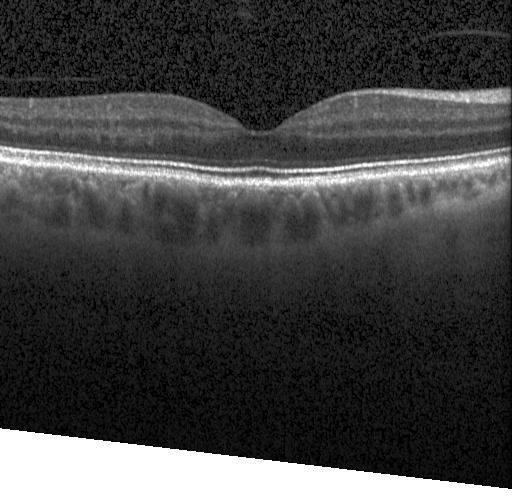

Finding: no choroidal neovascularization, diabetic macular edema, or drusen.